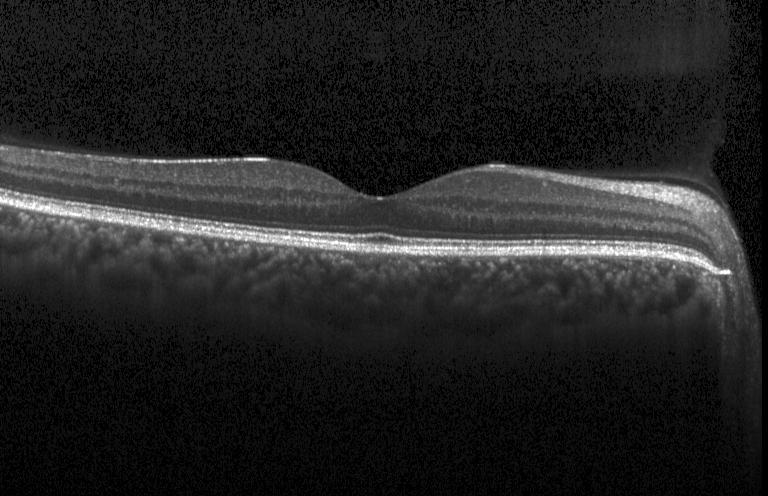

Spectral-domain optical coherence tomography. Heidelberg Spectralis OCT system. OCT B-scan.
Diagnosis: neither choroidal neovascularization, diabetic macular edema, nor drusen.